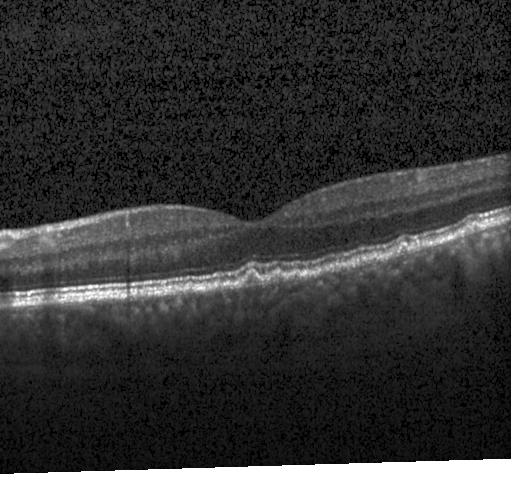

Dx: multiple drusen.